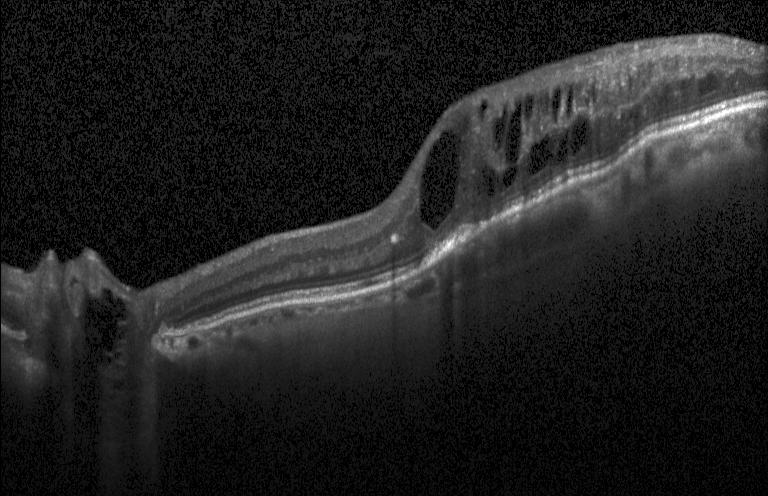

Spectral-domain OCT. Heidelberg Spectralis OCT system. Optical coherence tomography scan
This B-scan demonstrates diabetic macular edema (DME).